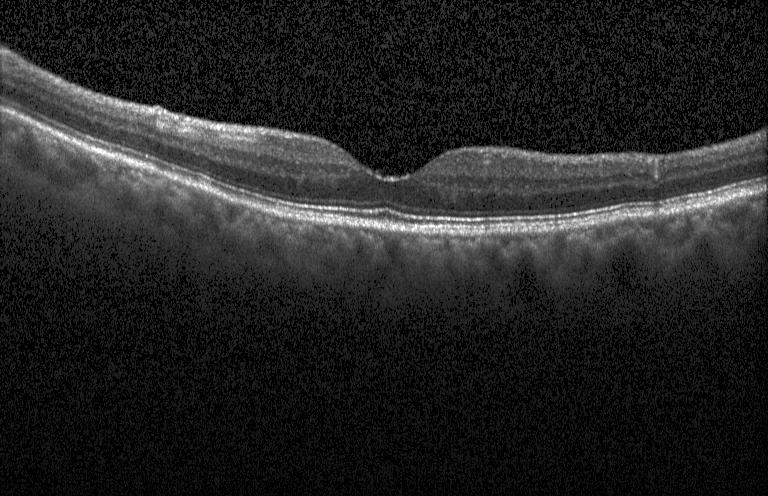
Retinal OCT cross-section. Horizontal scan through the fovea
Diagnosis: neither choroidal neovascularization, diabetic macular edema, nor drusen.